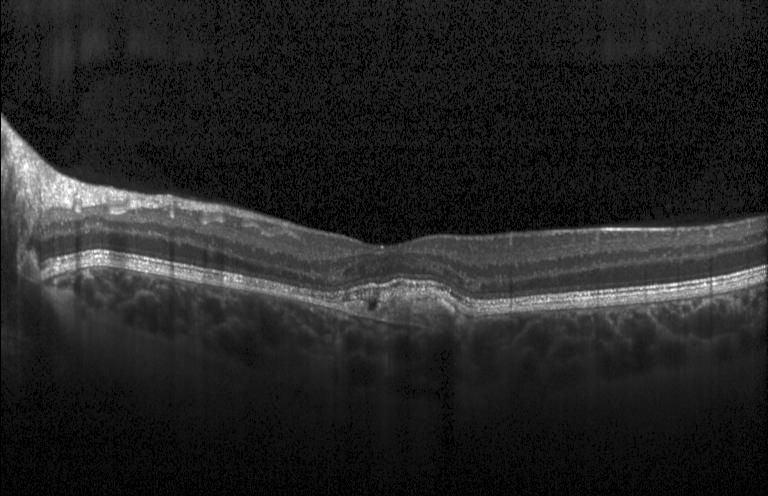 Optical coherence tomography scan · fovea-centered · spectral-domain OCT.
The scan shows CNV.